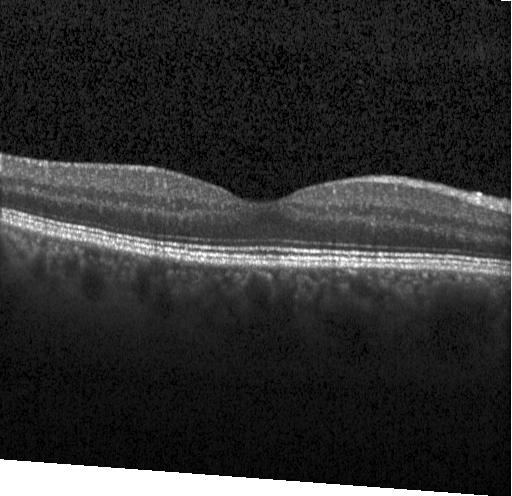

OCT line scan
Dx: no evidence of CNV, DME, or drusen.